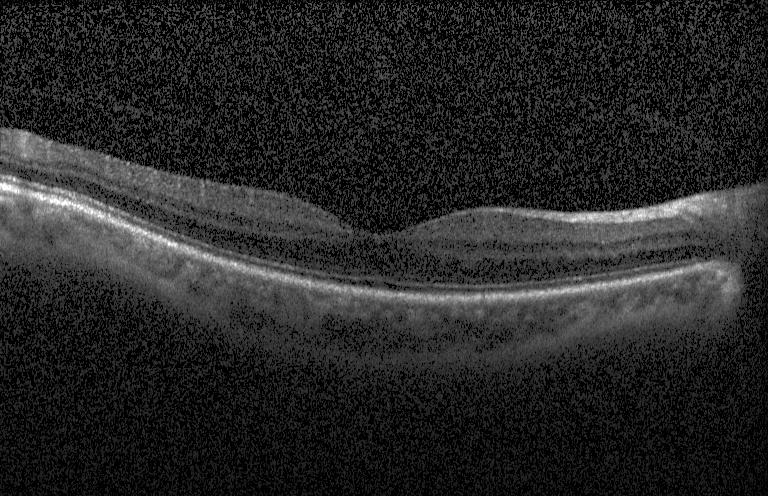 Acquired on a Heidelberg Spectralis, macular scan, retinal OCT cross-section
This B-scan demonstrates no evidence of CNV, DME, or drusen.